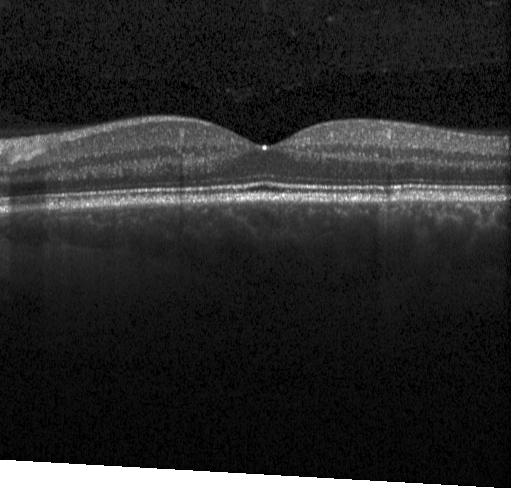 OCT B-scan — This B-scan demonstrates neither choroidal neovascularization, diabetic macular edema, nor drusen.